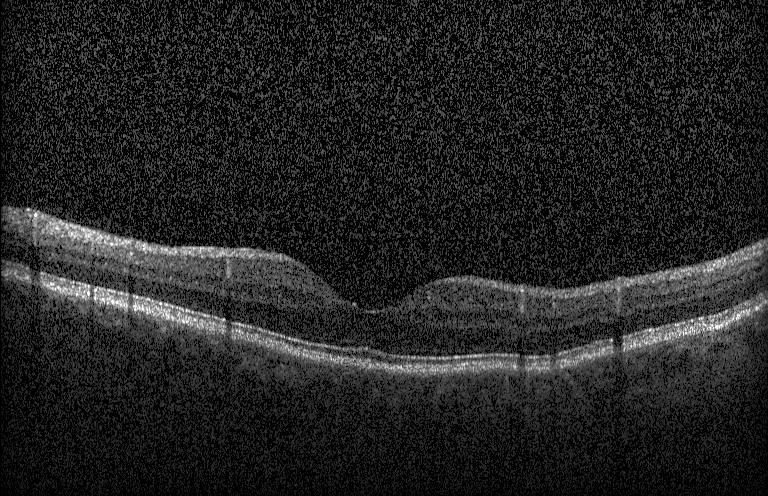 Centered on the fovea. OCT B-scan
Finding: no evidence of CNV, DME, or drusen.